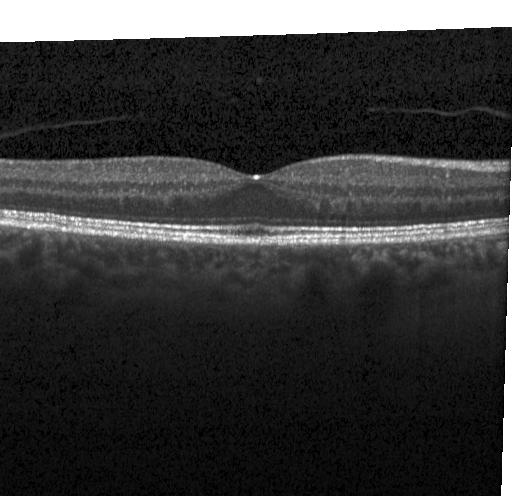 Heidelberg Spectralis OCT system. Retinal OCT B-scan — Diagnosis: no CNV, no DME, and no drusen.